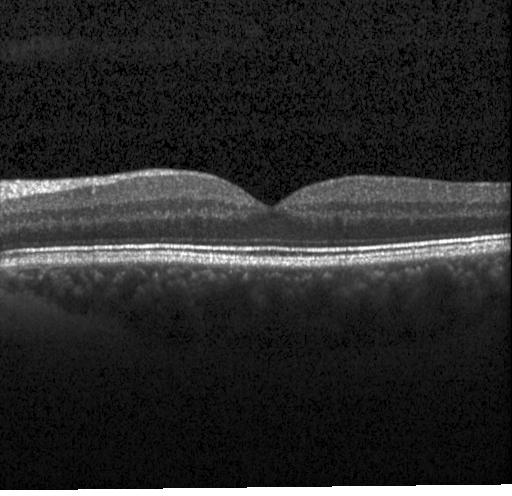

The scan shows neither CNV, DME, nor drusen.